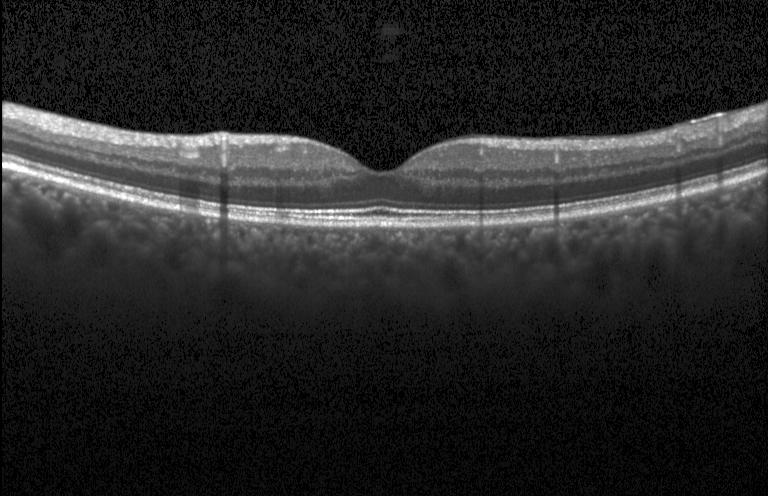 Diagnosis: no CNV, no DME, and no drusen.